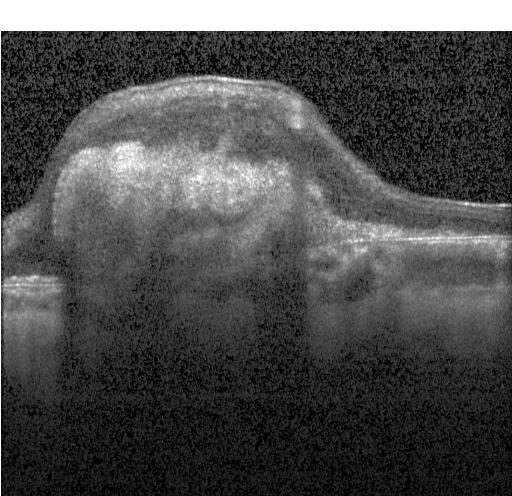

Optical coherence tomography scan, centered on the fovea, spectral-domain optical coherence tomography, acquired on a Heidelberg Spectralis
This B-scan demonstrates CNV.